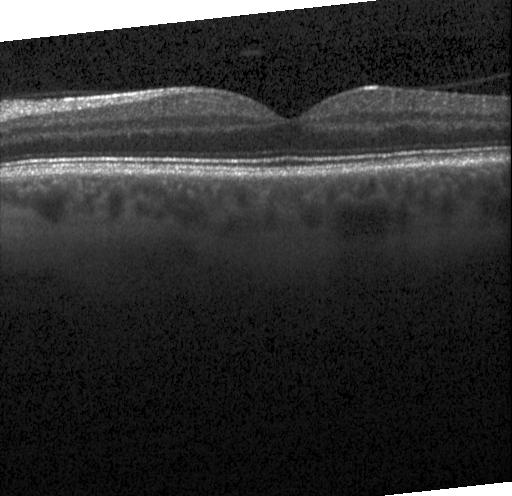

OCT scan showing neither choroidal neovascularization, diabetic macular edema, nor drusen.